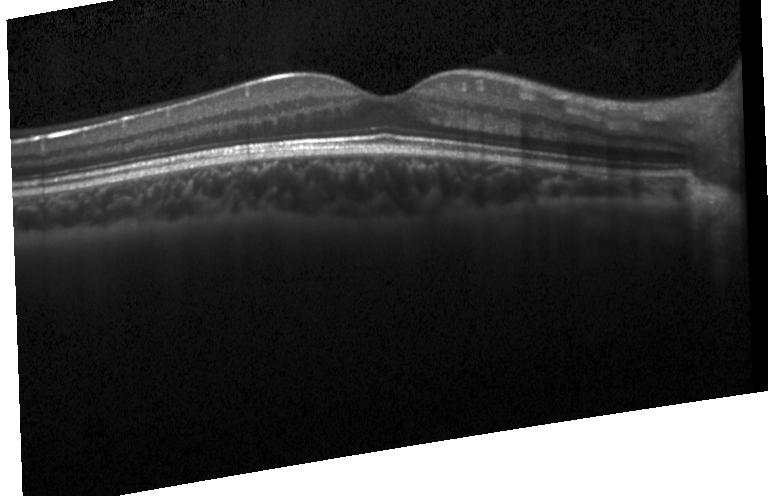
Instrument: Heidelberg Spectralis · fovea-centered · OCT line scan. Impression: no choroidal neovascularization, no diabetic macular edema, and no drusen.